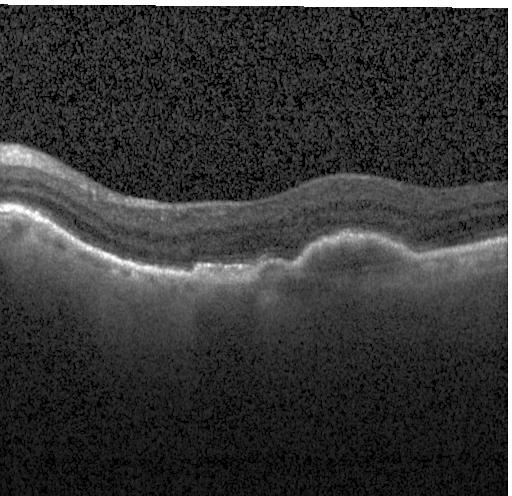 OCT B-scan showing a choroidal neovascular membrane.